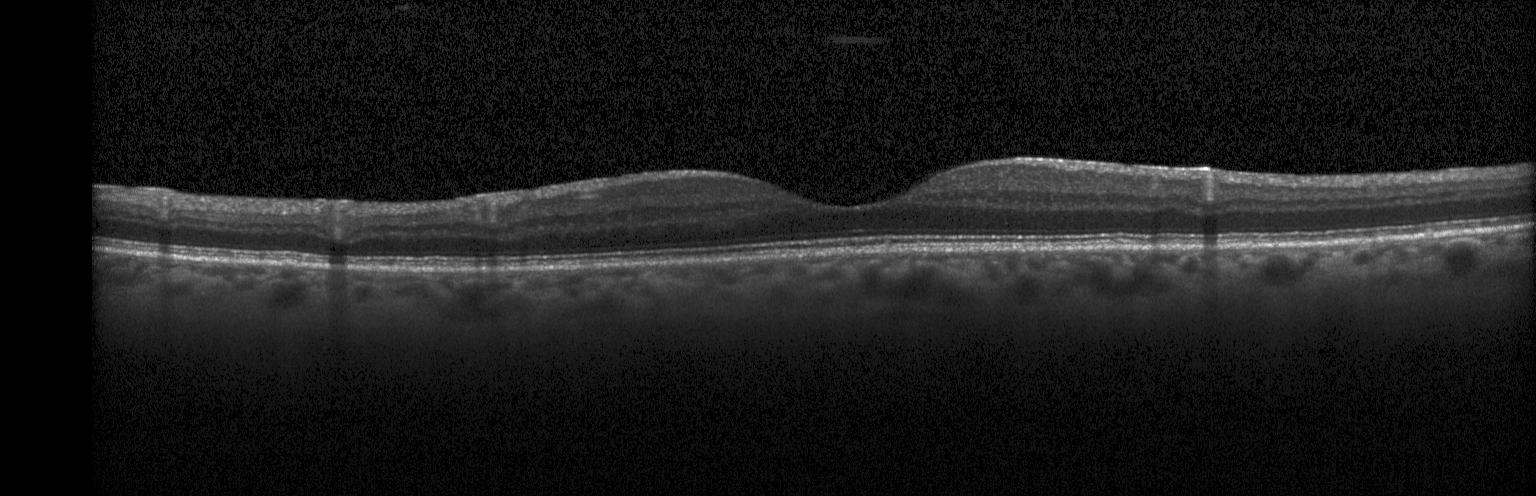 Optical coherence tomography B-scan. Through the macula — Finding: no evidence of choroidal neovascularization, diabetic macular edema, or drusen.